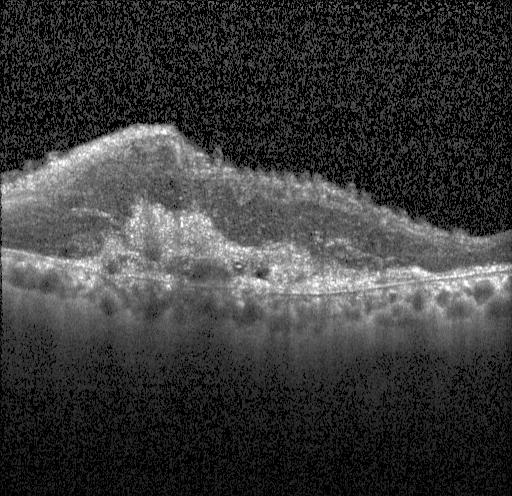
Finding: choroidal neovascularization (CNV).